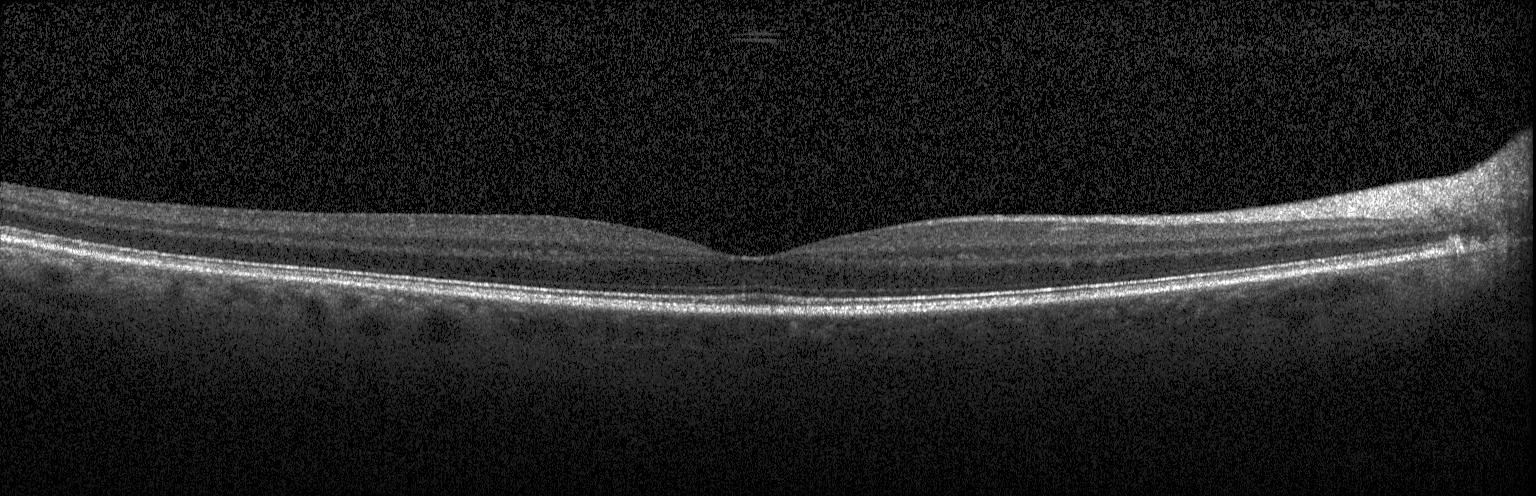

Optical coherence tomography scan.
Impression: no choroidal neovascularization, no diabetic macular edema, and no drusen.